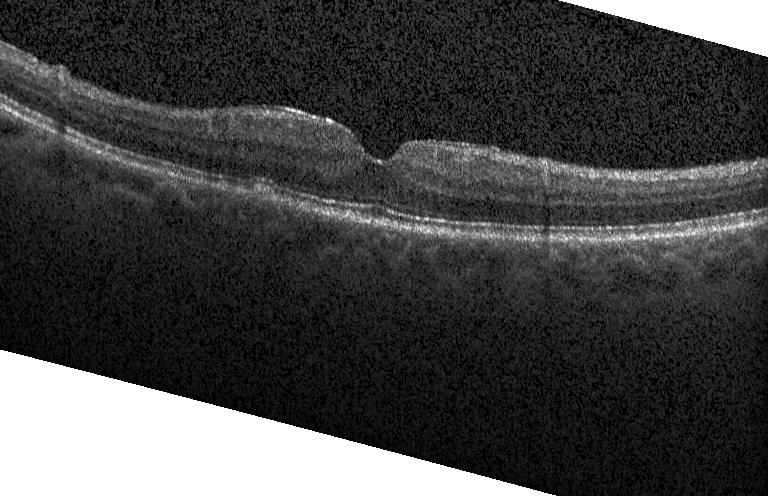
Macular scan, OCT line scan.
Diagnosis: sub-RPE drusenoid deposits.